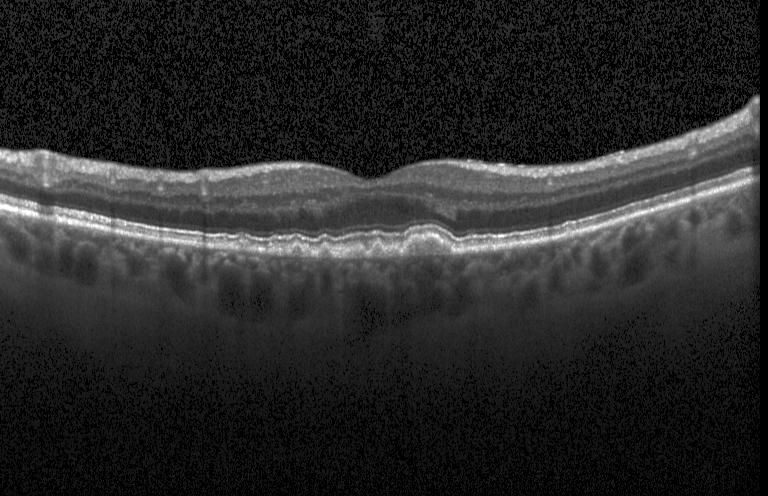

Optical coherence tomography B-scan, centered on the fovea.
Impression: sub-RPE drusenoid deposits.